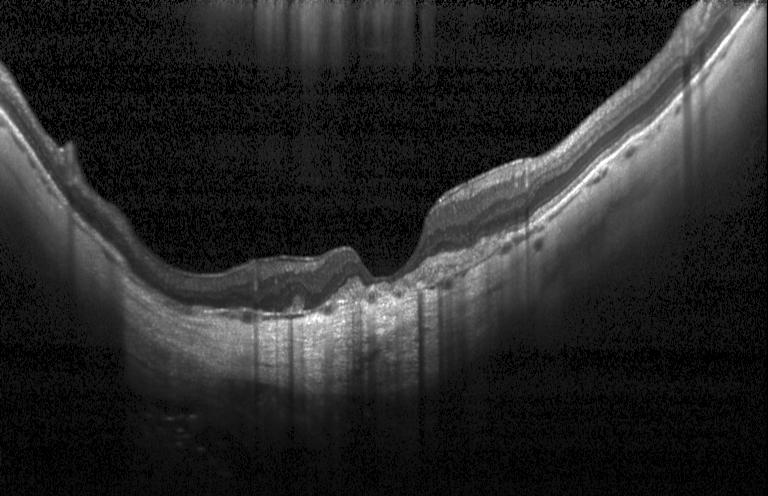
OCT line scan — Diagnosis: a choroidal neovascular membrane.